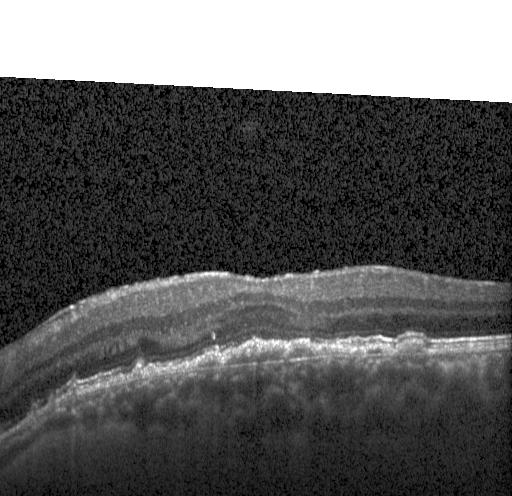 Retinal OCT B-scan.
Finding: choroidal neovascularization.